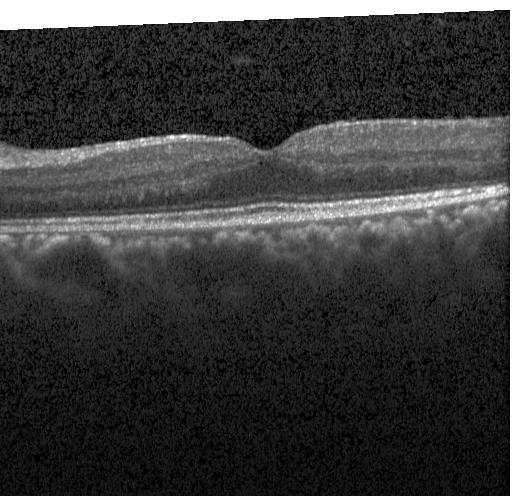

Assessment: DME.